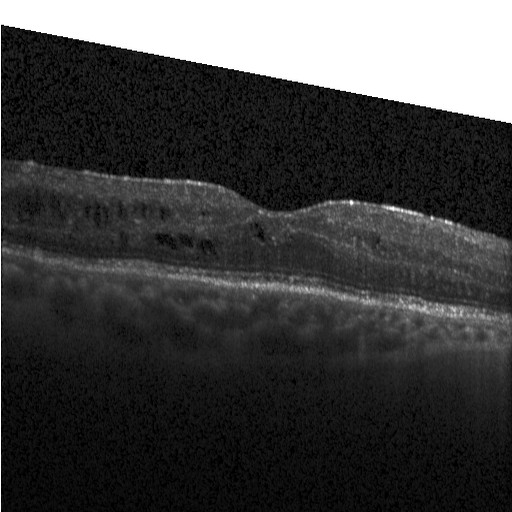

Finding: DME.